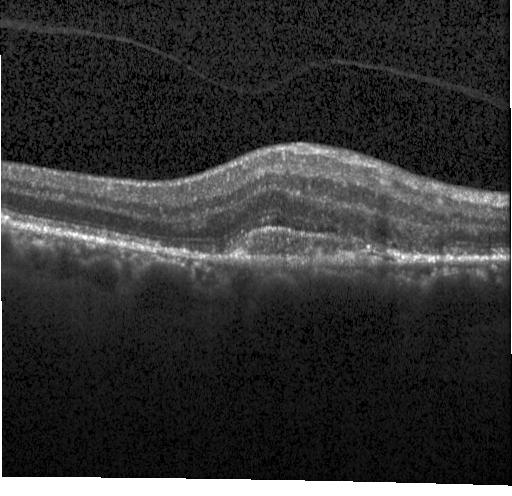 Diagnosis: CNV.